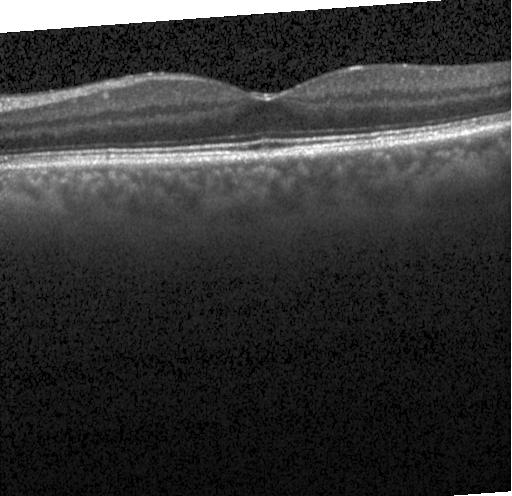

Finding: no choroidal neovascularization, no diabetic macular edema, and no drusen.